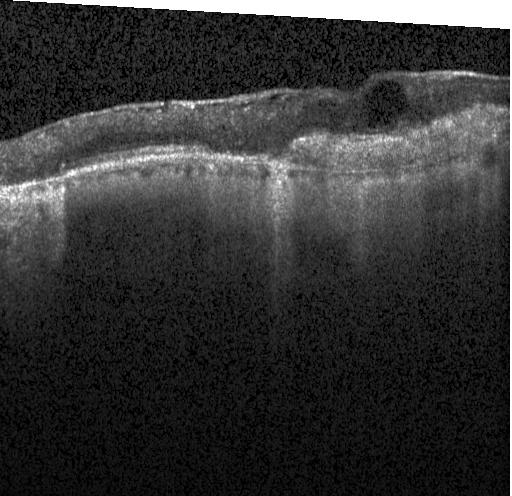 OCT line scan, through the macula, Heidelberg Spectralis — Impression: a choroidal neovascular membrane.